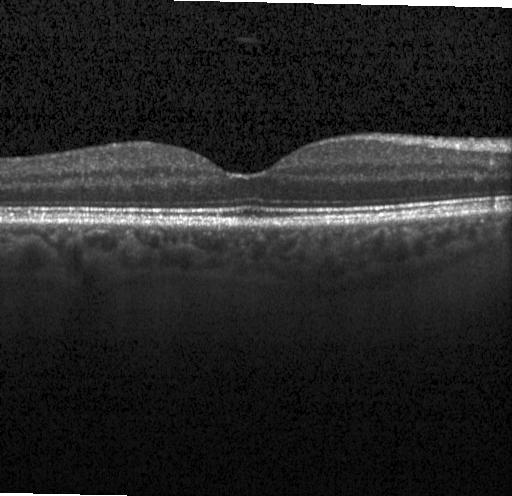 Impression: neither choroidal neovascularization, diabetic macular edema, nor drusen.